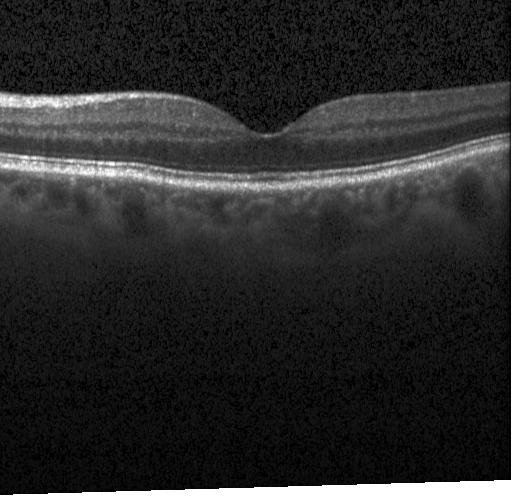

Spectral-domain optical coherence tomography; optical coherence tomography B-scan; horizontal scan through the fovea; Heidelberg Spectralis OCT system. No choroidal neovascularization, diabetic macular edema, or drusen.